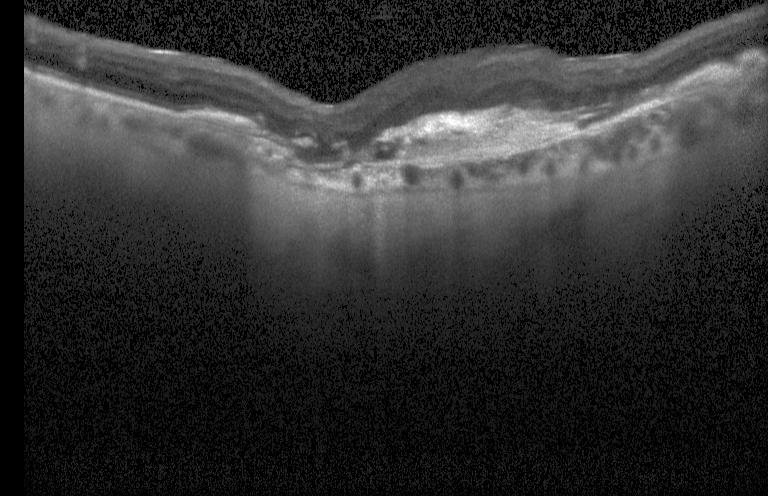
Optical coherence tomography B-scan — Assessment: a choroidal neovascular membrane.